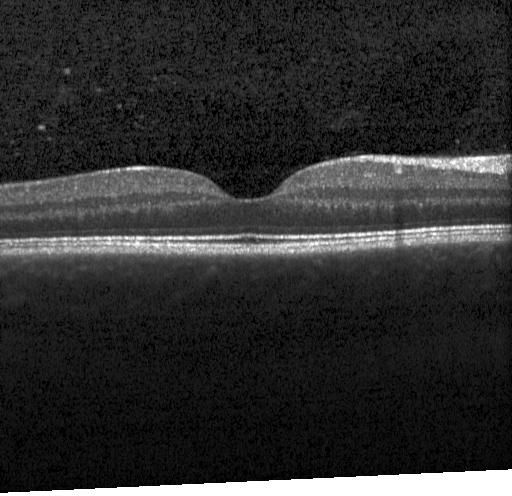
OCT line scan. Acquired on a Heidelberg Spectralis. Fovea-centered. Impression: no evidence of CNV, DME, or drusen.